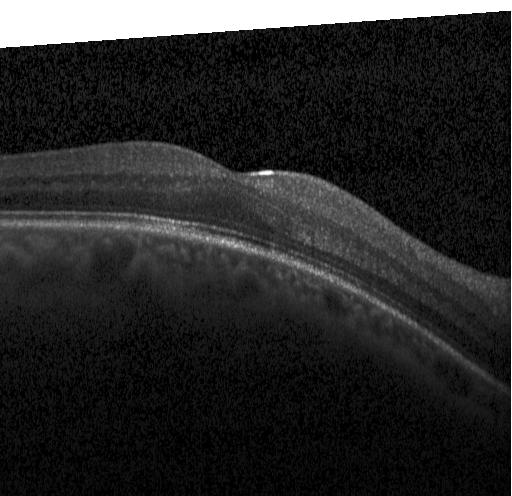

OCT B-scan.
Finding: no CNV, DME, or drusen.